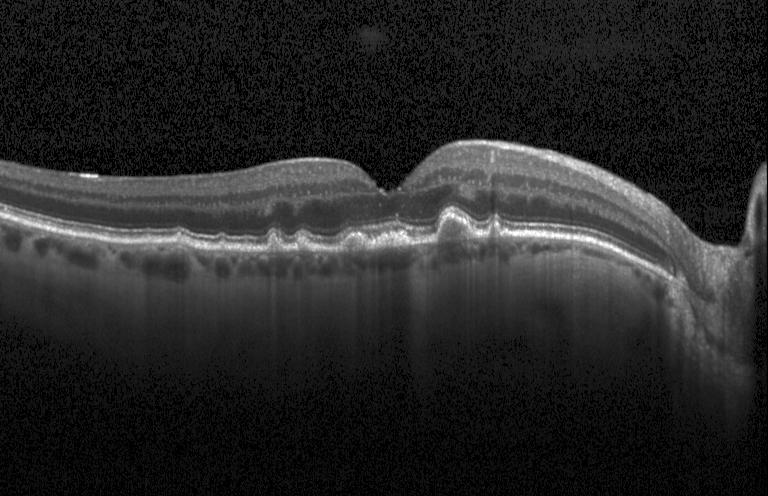
Centered on the fovea; Heidelberg Spectralis; OCT line scan; spectral-domain optical coherence tomography
Diagnosis: sub-RPE drusenoid deposits.